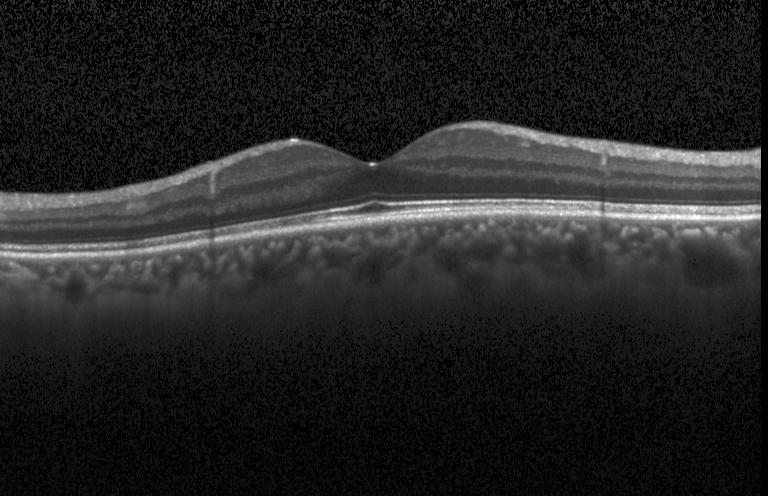
Retinal OCT cross-section showing neither choroidal neovascularization, diabetic macular edema, nor drusen.